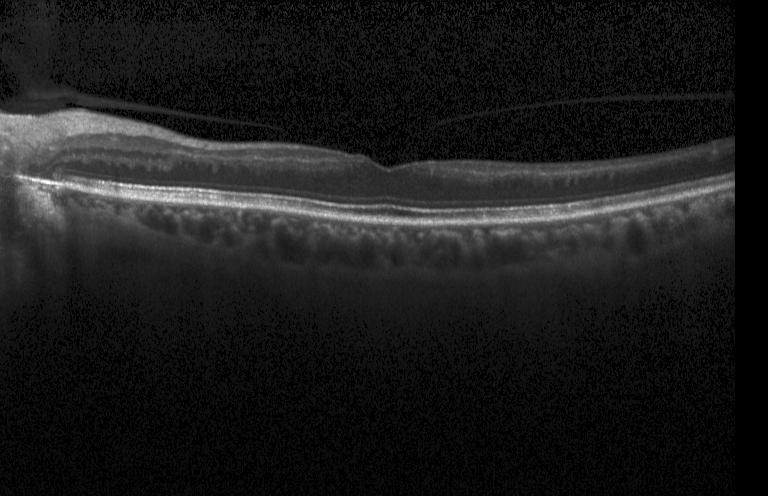
Optical coherence tomography B-scan. Spectral-domain optical coherence tomography. Heidelberg Spectralis OCT system. Centered on the fovea
Impression: no evidence of choroidal neovascularization, diabetic macular edema, or drusen.